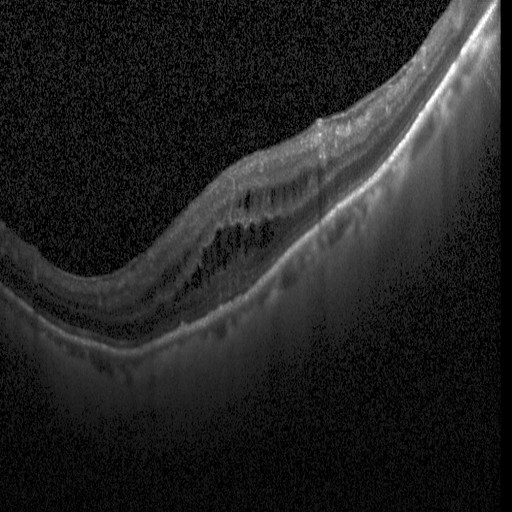
OCT line scan — DME.